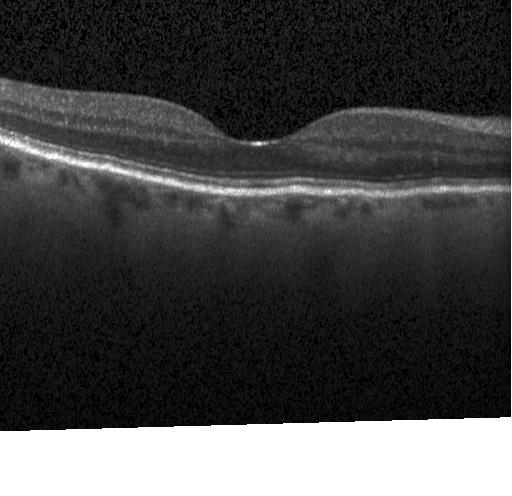
OCT finding: no CNV, DME, or drusen.